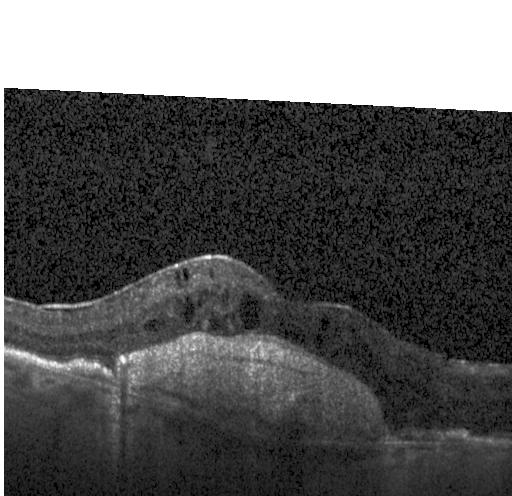 Impression: a choroidal neovascular membrane.